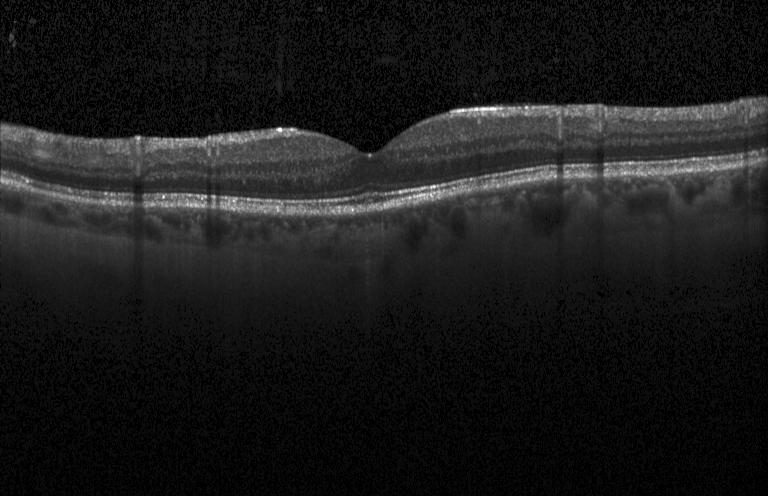

OCT line scan. Instrument: Heidelberg Spectralis. Spectral-domain OCT. Through the macula. This B-scan demonstrates neither choroidal neovascularization, diabetic macular edema, nor drusen.